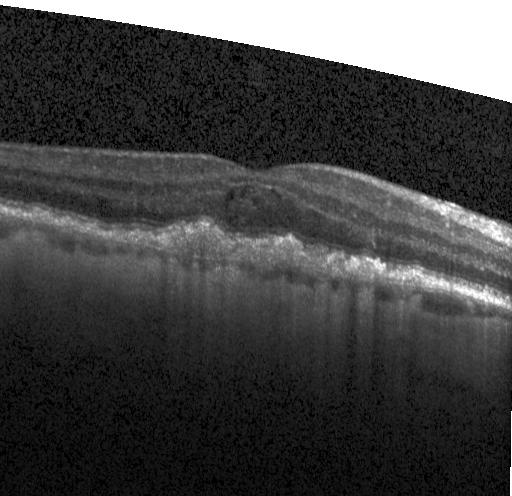

OCT line scan. A choroidal neovascular membrane.